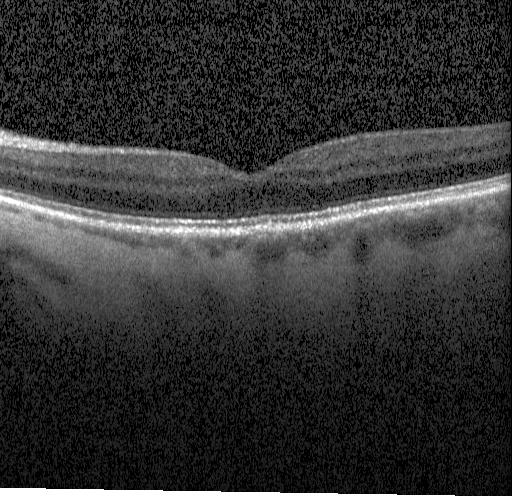 Retinal OCT B-scan · SD-OCT.
Dx: no choroidal neovascularization, no diabetic macular edema, and no drusen.